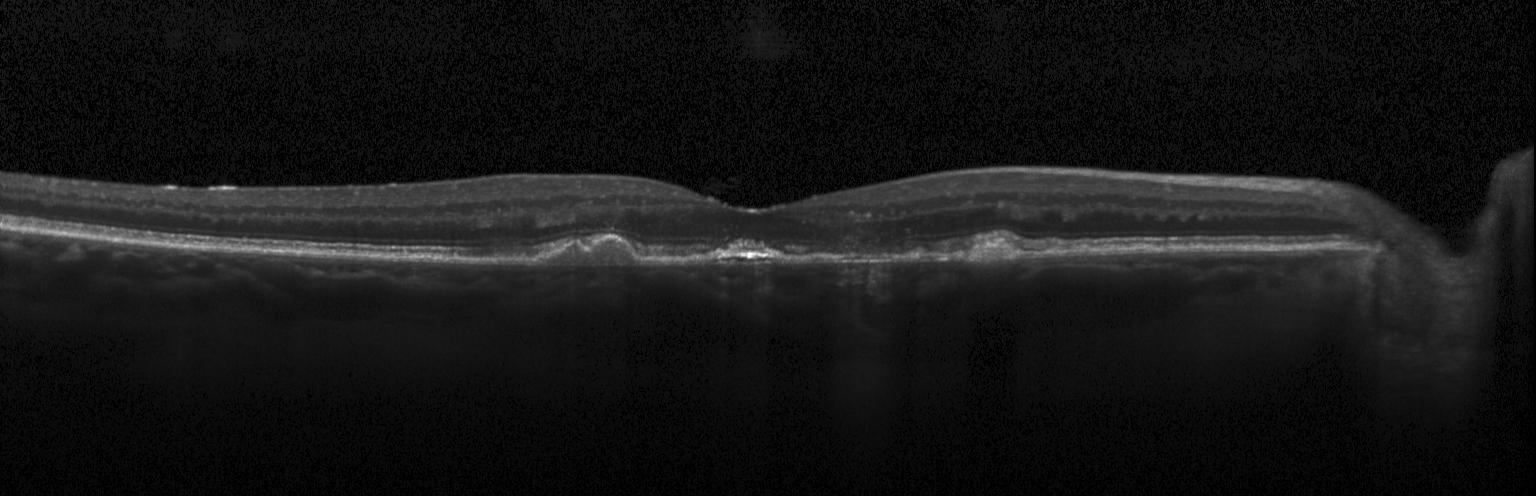 Optical coherence tomography scan · SD-OCT · horizontal scan through the fovea · acquired on a Heidelberg Spectralis. Impression: a choroidal neovascular membrane.